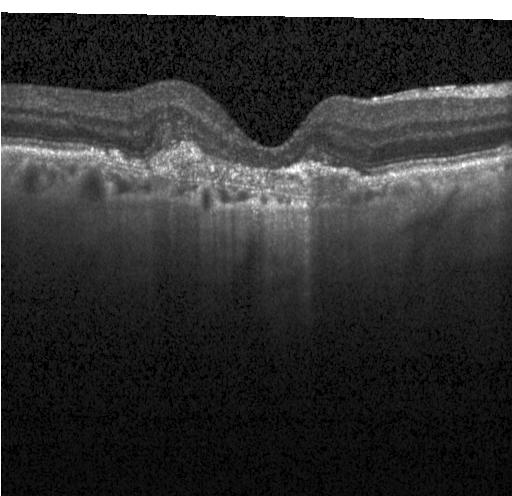
OCT scan showing choroidal neovascularization.